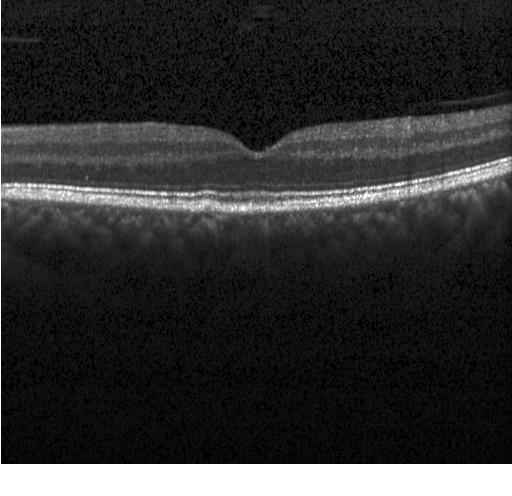 Retinal OCT cross-section. OCT finding: sub-RPE drusenoid deposits.